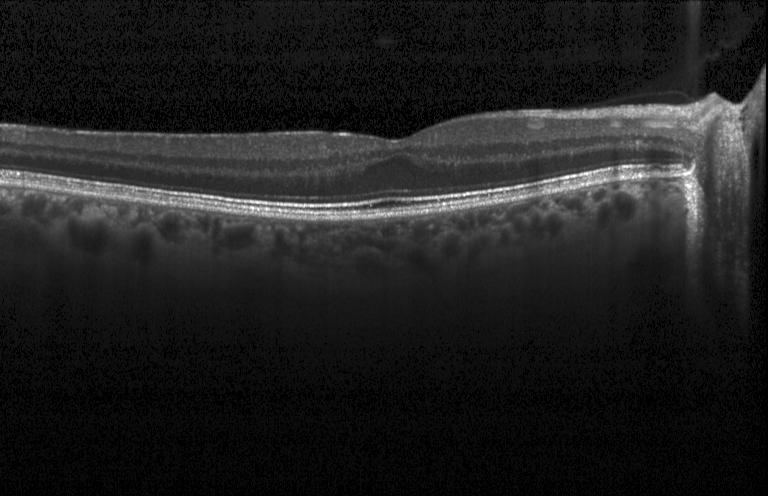

This B-scan demonstrates no evidence of choroidal neovascularization, diabetic macular edema, or drusen.